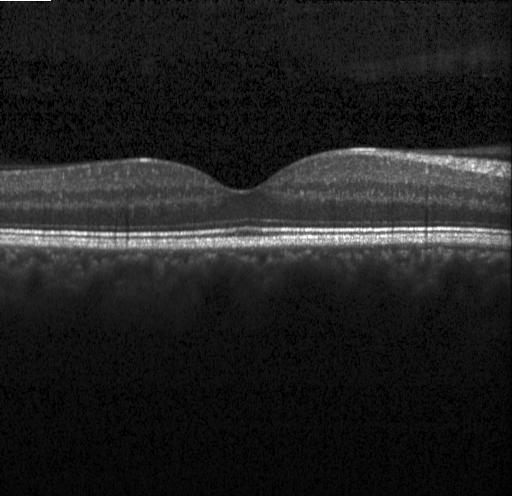 Diagnosis: no choroidal neovascularization, no diabetic macular edema, and no drusen.